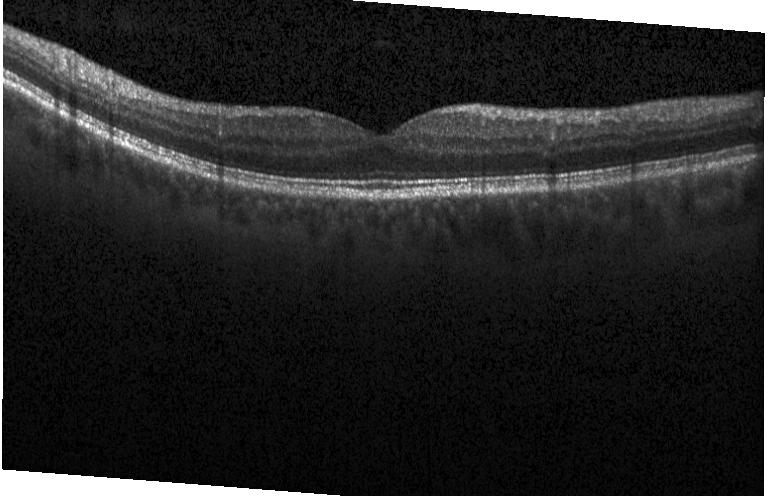 Impression: neither CNV, DME, nor drusen.